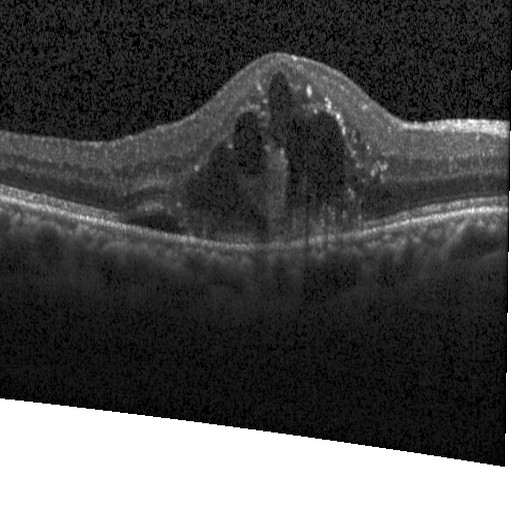
OCT line scan · spectral-domain OCT · instrument: Heidelberg Spectralis — Dx: DME.